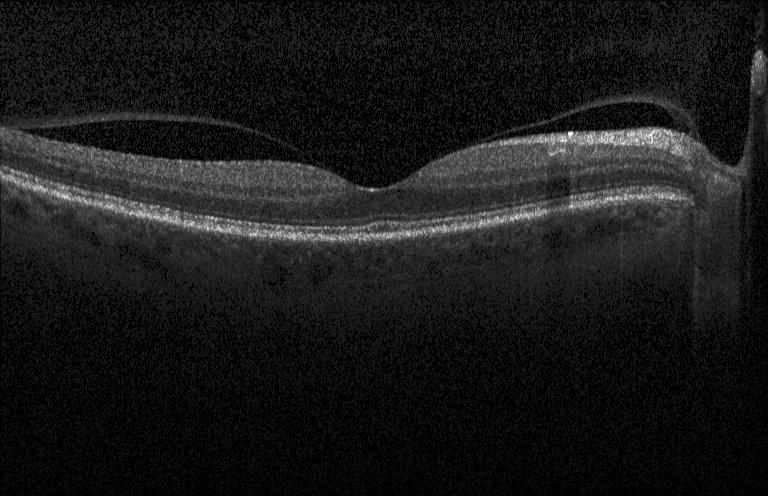

OCT line scan
OCT finding: neither choroidal neovascularization, diabetic macular edema, nor drusen.